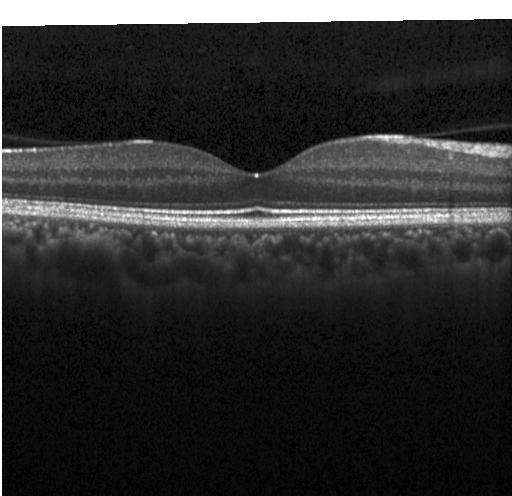

SD-OCT, retinal OCT B-scan.
Impression: no choroidal neovascularization, no diabetic macular edema, and no drusen.